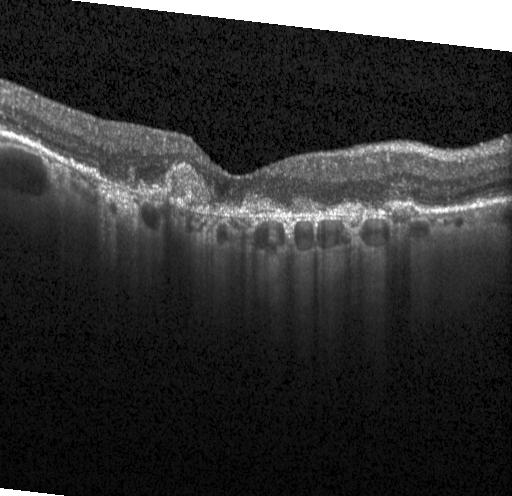

Retinal OCT cross-section; centered on the fovea.
Choroidal neovascularization (CNV).